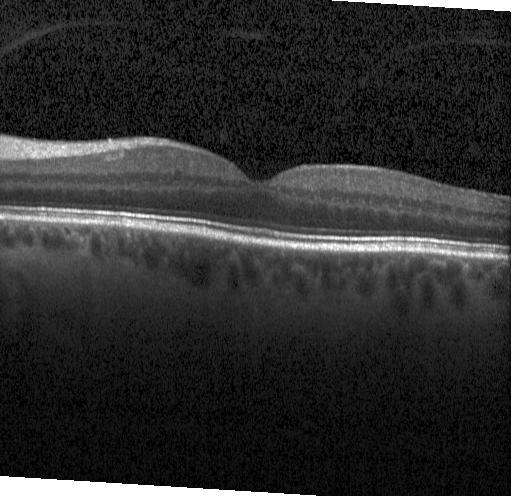
Retinal OCT cross-section showing no evidence of choroidal neovascularization, diabetic macular edema, or drusen.